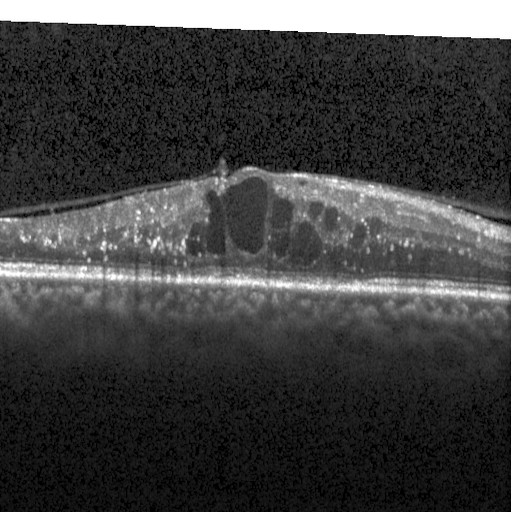
OCT line scan
Impression: DME.